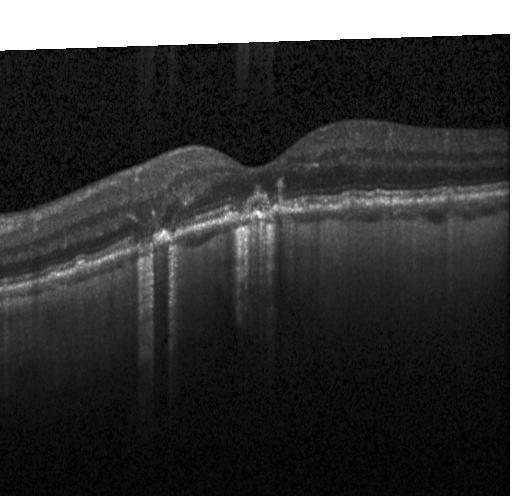
Acquired on a Heidelberg Spectralis; OCT line scan; centered on the fovea; spectral-domain optical coherence tomography. Macular OCT: CNV.